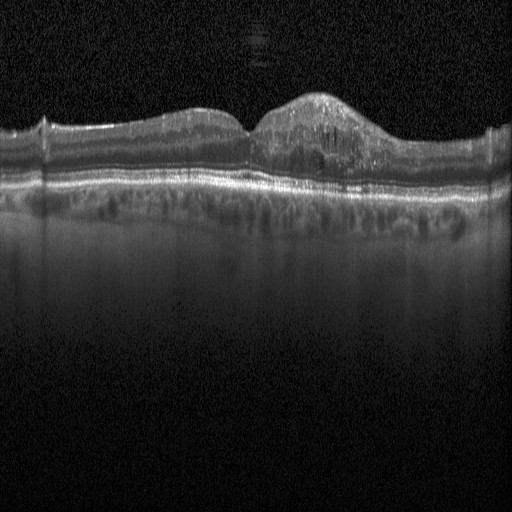
The scan shows DME.